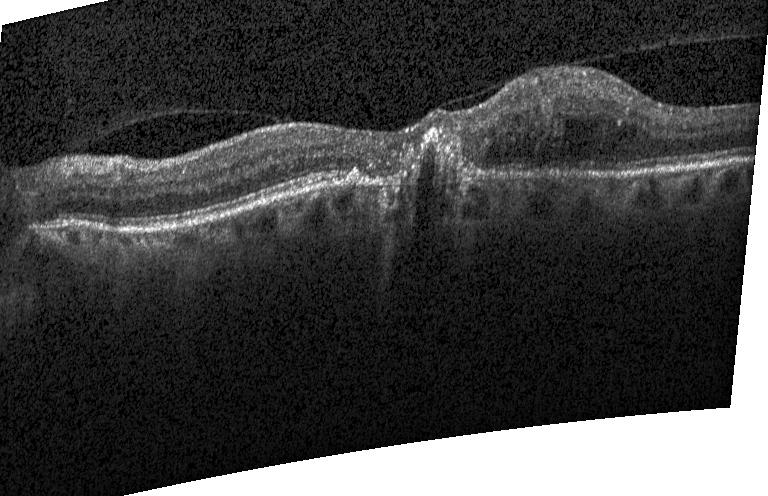 Acquired on a Heidelberg Spectralis. Macular scan. Spectral-domain optical coherence tomography. OCT B-scan.
Diagnosis: a choroidal neovascular membrane.